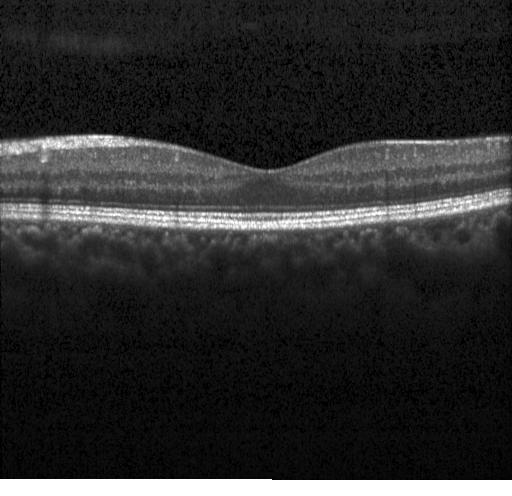

OCT scan showing no CNV, DME, or drusen.